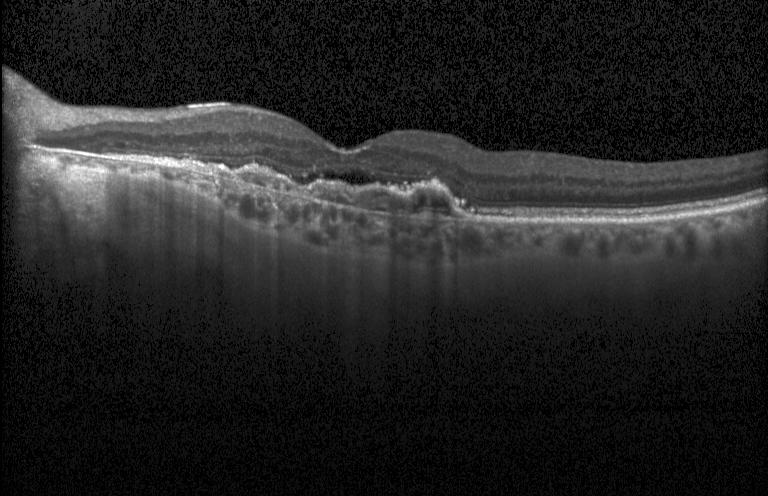
This B-scan demonstrates a choroidal neovascular membrane.